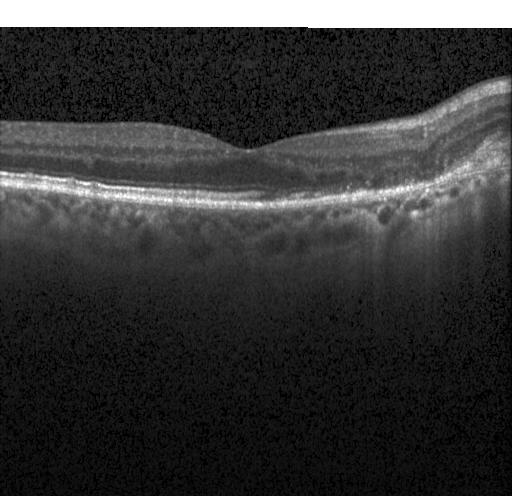
Retinal OCT cross-section showing a choroidal neovascular membrane.